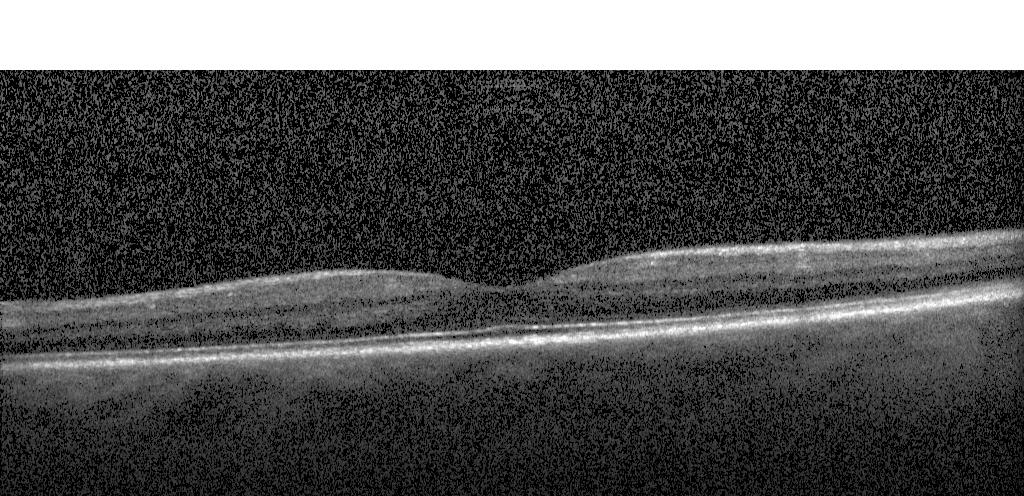 Dx: no CNV, no DME, and no drusen.